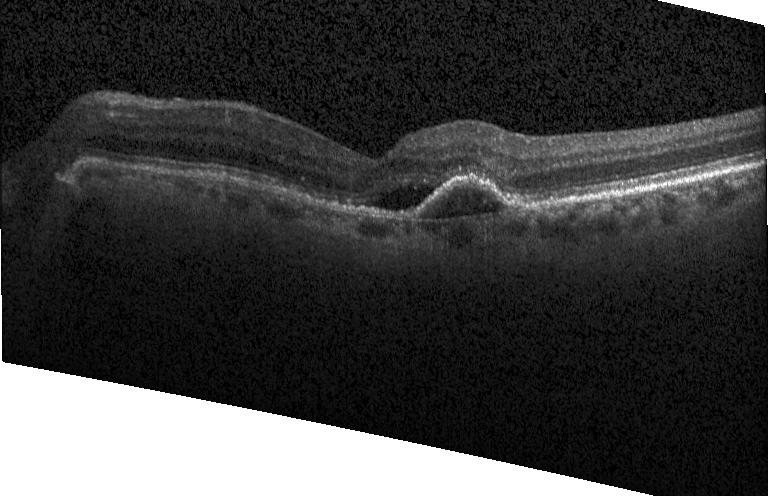

Spectral-domain optical coherence tomography · acquired on a Heidelberg Spectralis · OCT B-scan · through the macula. Choroidal neovascularization (CNV).